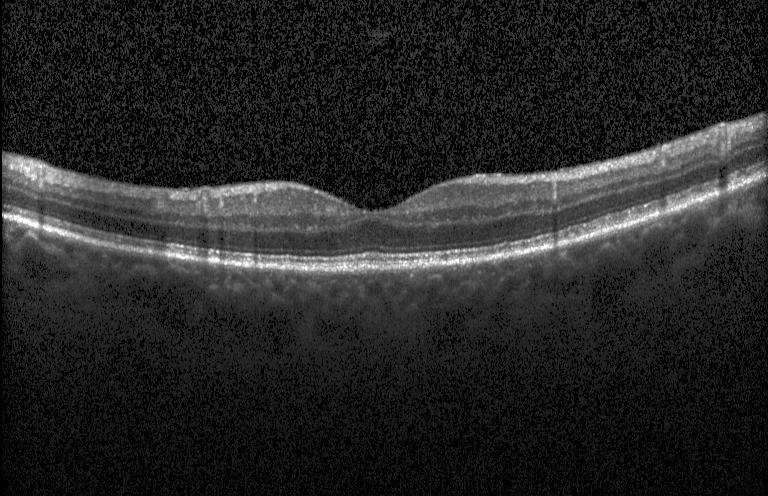
Retinal OCT cross-section — Finding: no evidence of choroidal neovascularization, diabetic macular edema, or drusen.